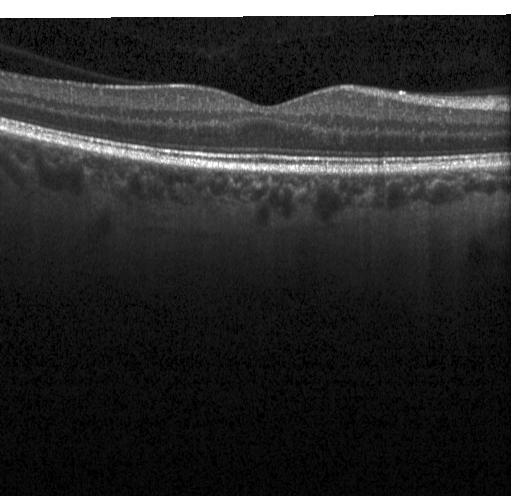 Heidelberg Spectralis, SD-OCT, fovea-centered, OCT line scan — The scan shows neither CNV, DME, nor drusen.